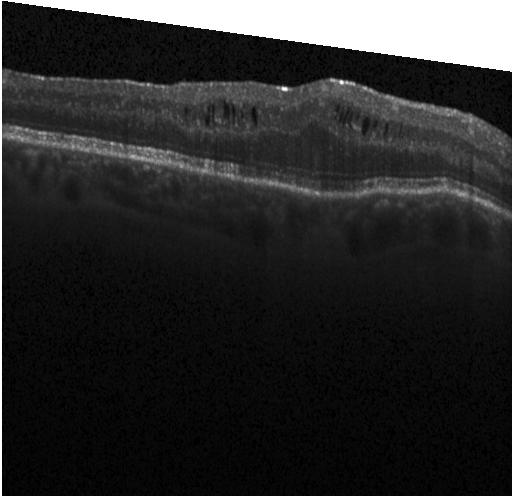

Retinal OCT cross-section
OCT finding: diabetic macular edema.